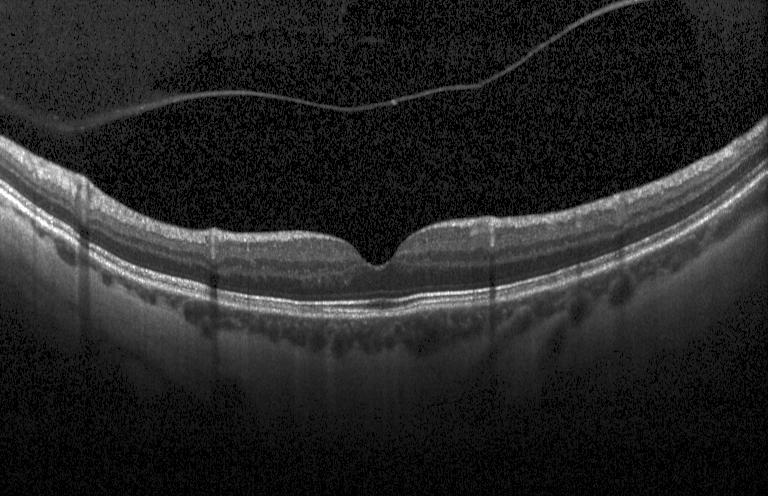 Diagnosis: neither choroidal neovascularization, diabetic macular edema, nor drusen.